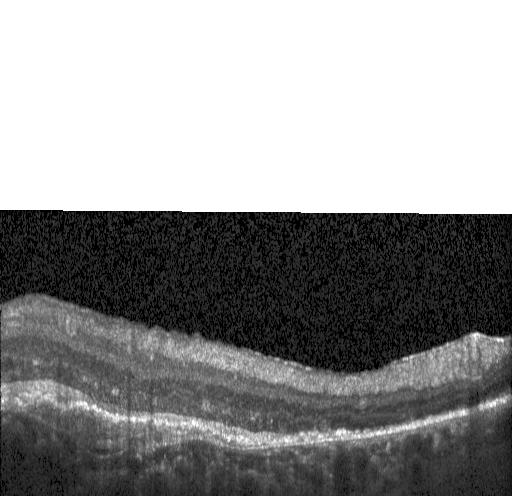

Optical coherence tomography scan; fovea-centered
Diagnosis: choroidal neovascularization (CNV).